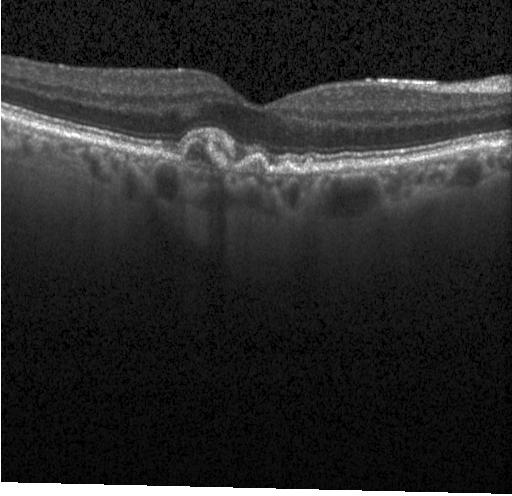 Spectral-domain optical coherence tomography · fovea-centered · retinal OCT B-scan · Heidelberg Spectralis OCT system — Diagnosis: a choroidal neovascular membrane.